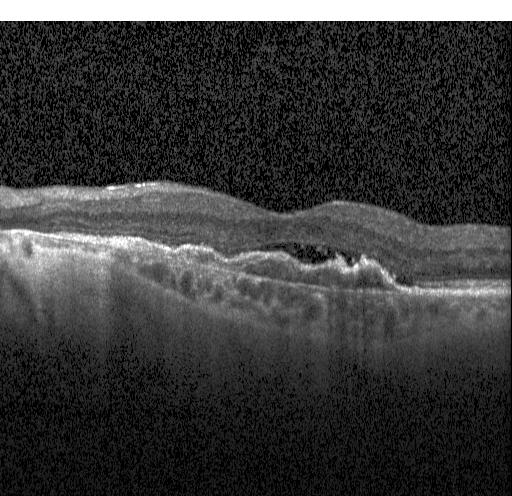
Optical coherence tomography B-scan
Finding: CNV.